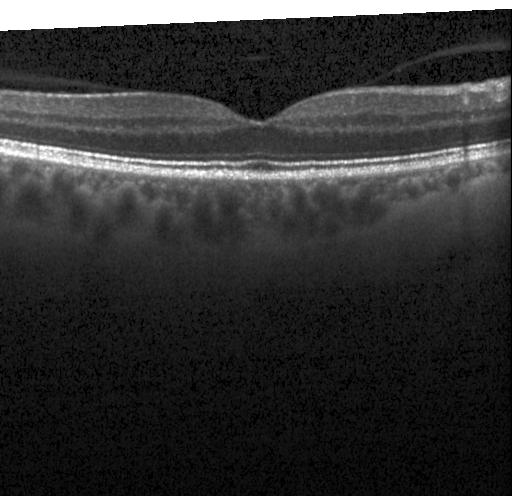 Retinal OCT B-scan — OCT finding: no CNV, no DME, and no drusen.